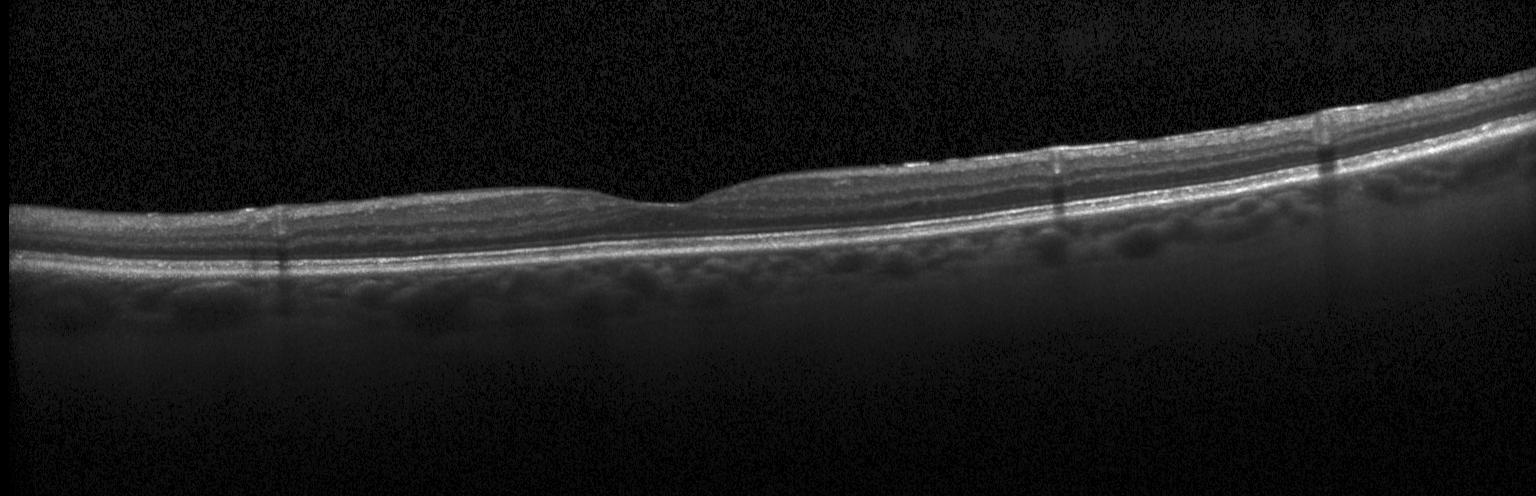
The scan shows no evidence of choroidal neovascularization, diabetic macular edema, or drusen.